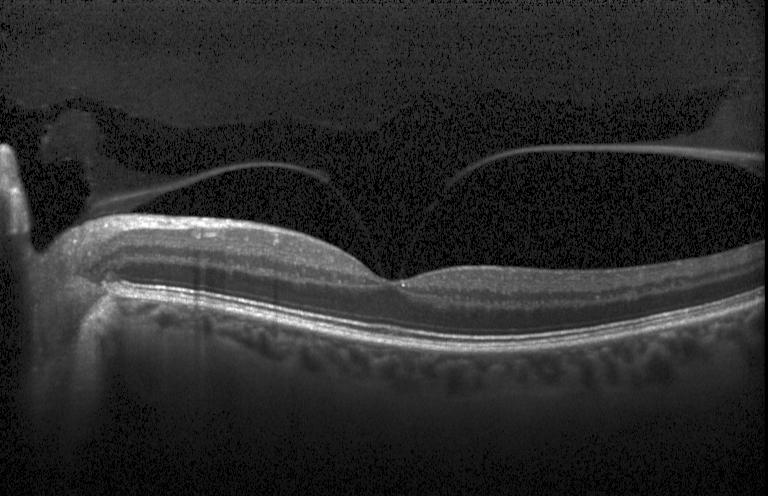
Impression: no CNV, DME, or drusen.